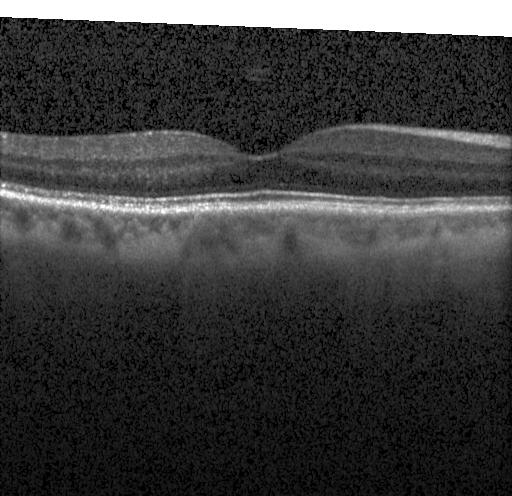

Retinal OCT cross-section. Diagnosis: no evidence of CNV, DME, or drusen.